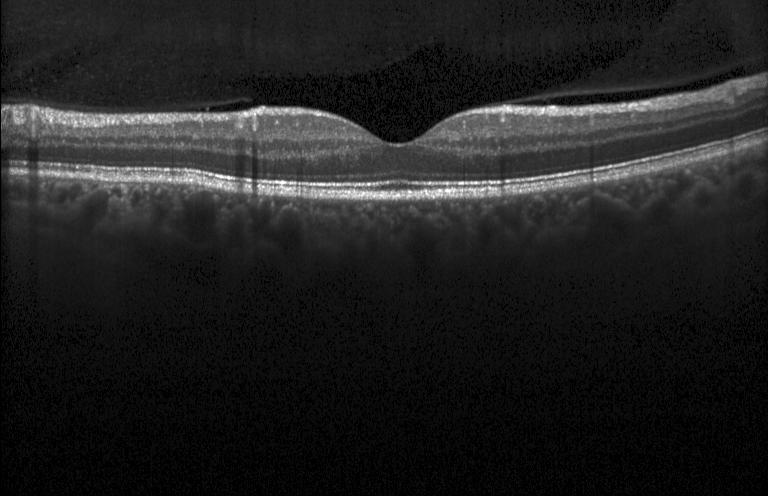 Finding: no CNV, DME, or drusen.